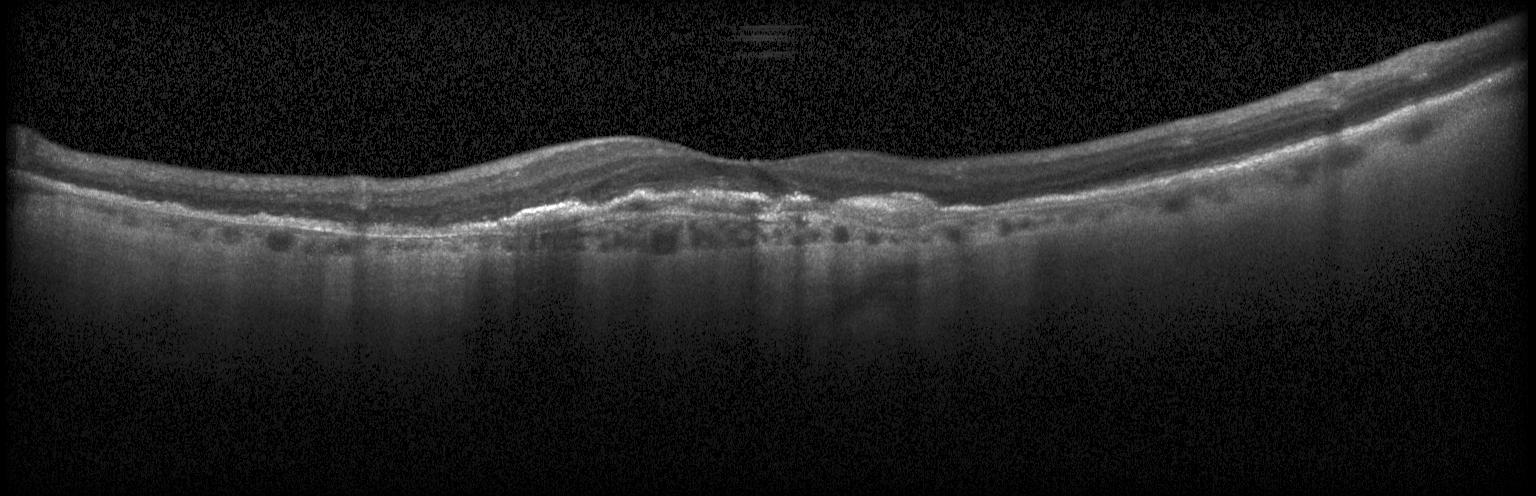
OCT finding: choroidal neovascularization (CNV).